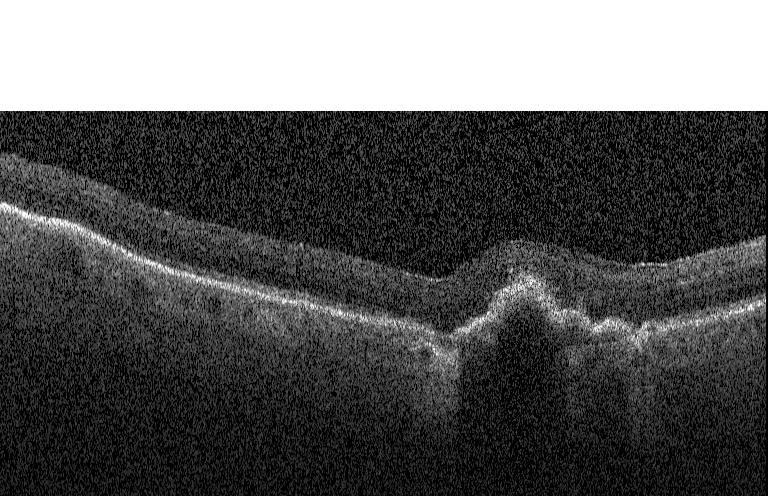

OCT B-scan · acquired on a Heidelberg Spectralis · centered on the fovea · spectral-domain optical coherence tomography.
Finding: CNV.